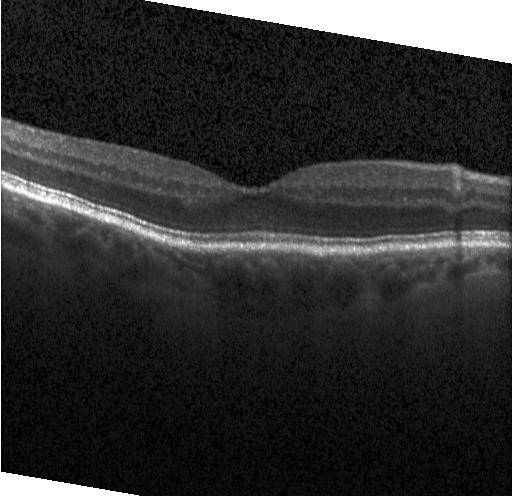

Assessment: no evidence of choroidal neovascularization, diabetic macular edema, or drusen.